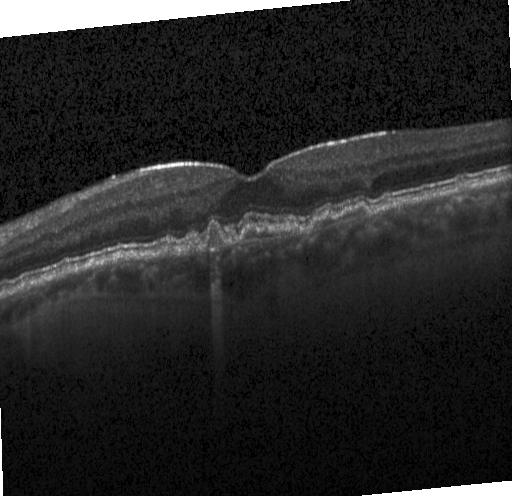

Horizontal scan through the fovea; OCT B-scan. Assessment: drusen.